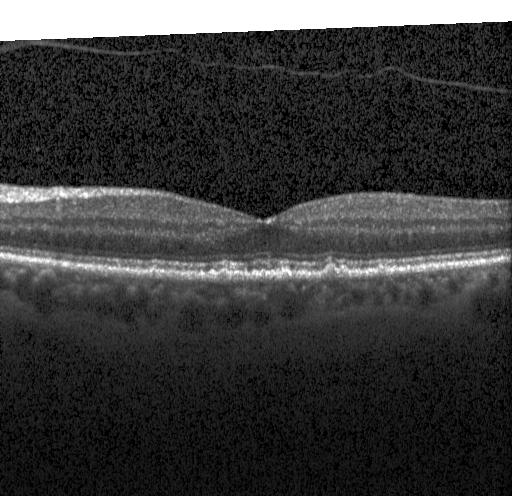 Spectral-domain OCT; optical coherence tomography B-scan; instrument: Heidelberg Spectralis — This B-scan demonstrates multiple drusen.